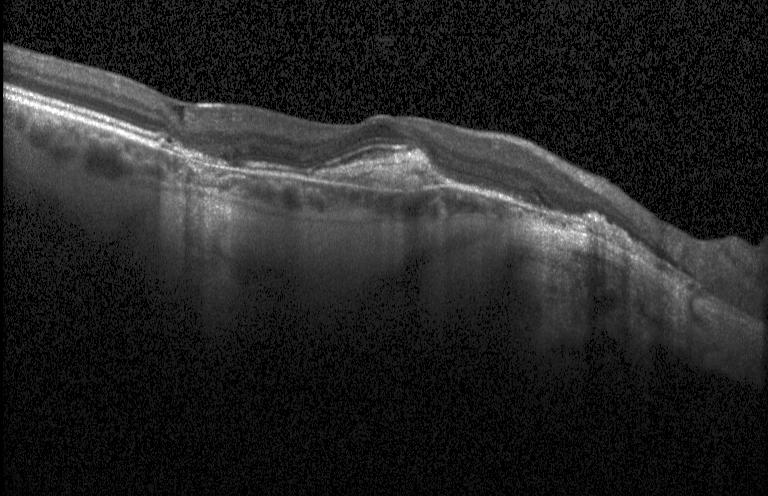

Horizontal scan through the fovea, optical coherence tomography B-scan, SD-OCT, instrument: Heidelberg Spectralis.
This B-scan demonstrates a choroidal neovascular membrane.